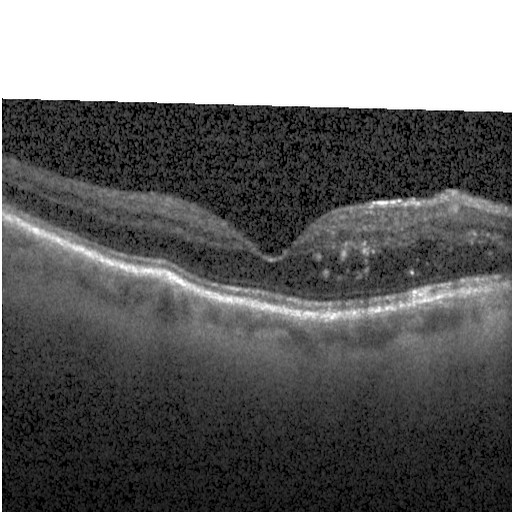 Macular scan. Spectral-domain OCT. Optical coherence tomography B-scan. Diagnosis: diabetic macular edema.